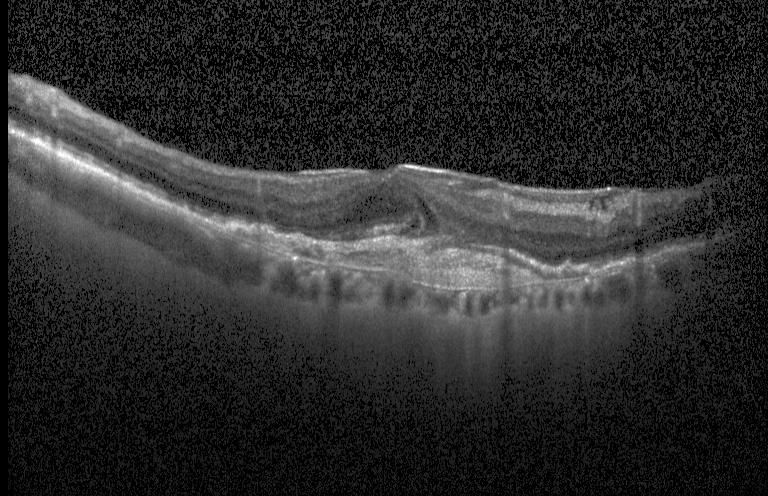 SD-OCT. Instrument: Heidelberg Spectralis. Optical coherence tomography B-scan. Centered on the fovea
Impression: choroidal neovascularization (CNV).